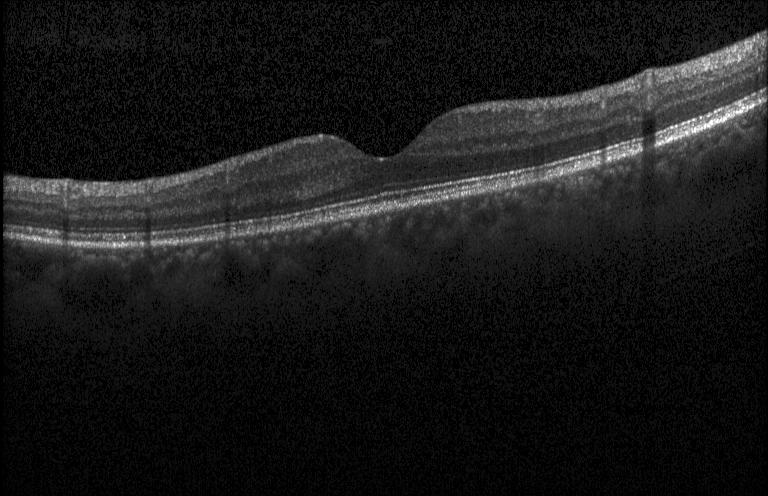

Macular OCT demonstrating no choroidal neovascularization, no diabetic macular edema, and no drusen.